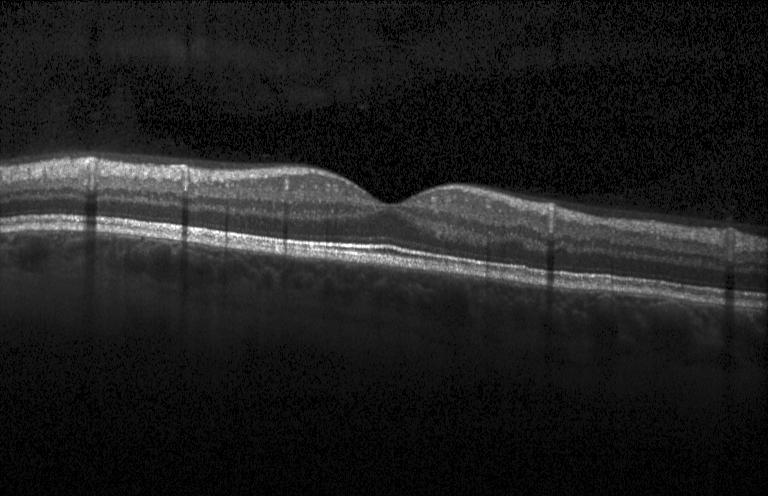
Dx: no evidence of CNV, DME, or drusen.